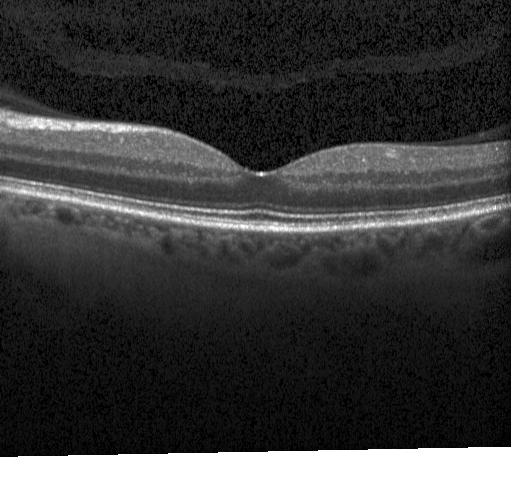 Impression: no evidence of choroidal neovascularization, diabetic macular edema, or drusen.